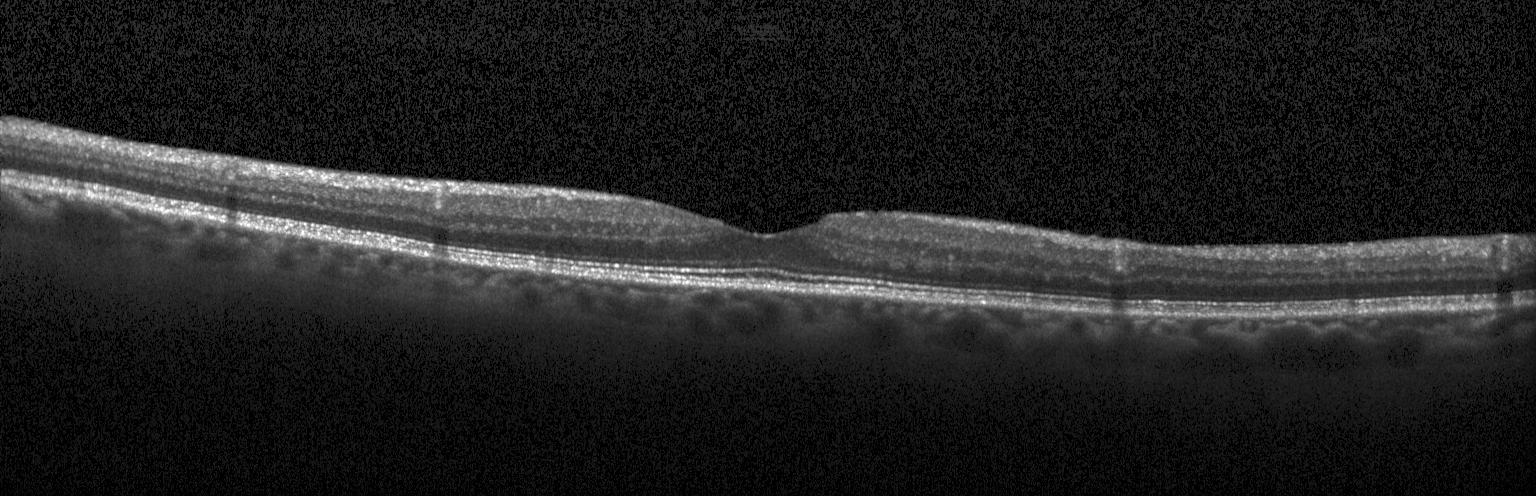 Optical coherence tomography B-scan. The scan shows no choroidal neovascularization, no diabetic macular edema, and no drusen.